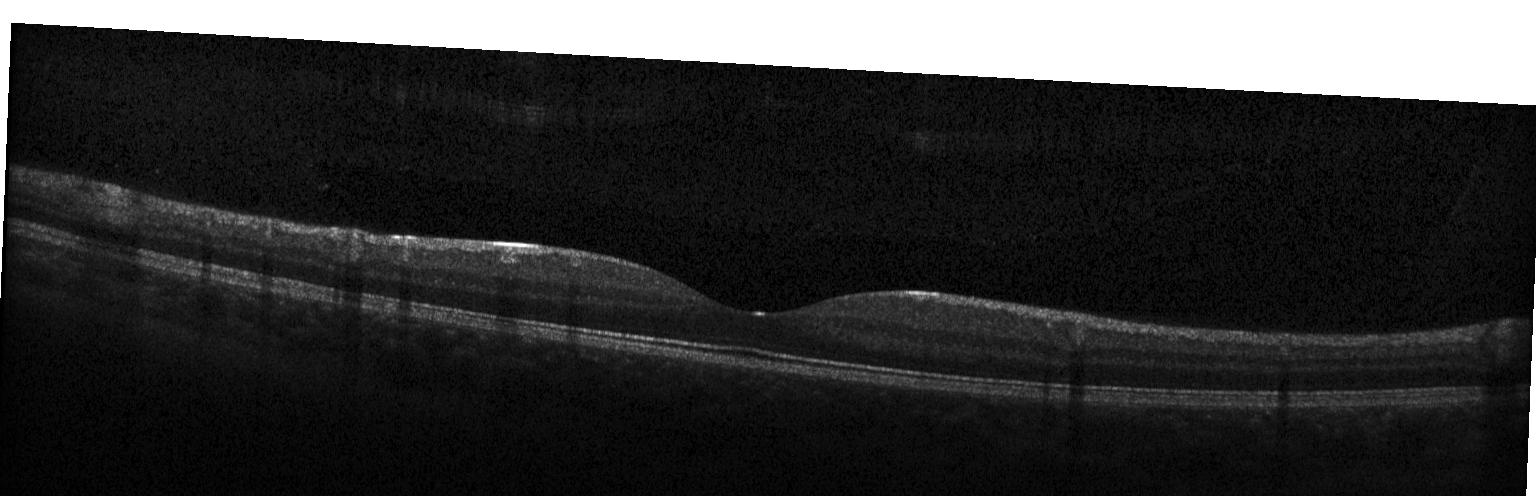

Retinal OCT cross-section, spectral-domain OCT
Assessment: neither choroidal neovascularization, diabetic macular edema, nor drusen.